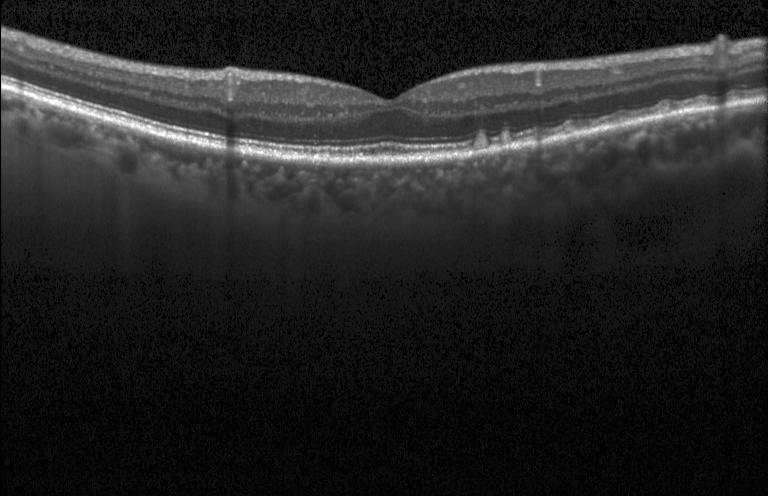
Spectral-domain OCT. Optical coherence tomography B-scan
This B-scan demonstrates sub-RPE drusenoid deposits.